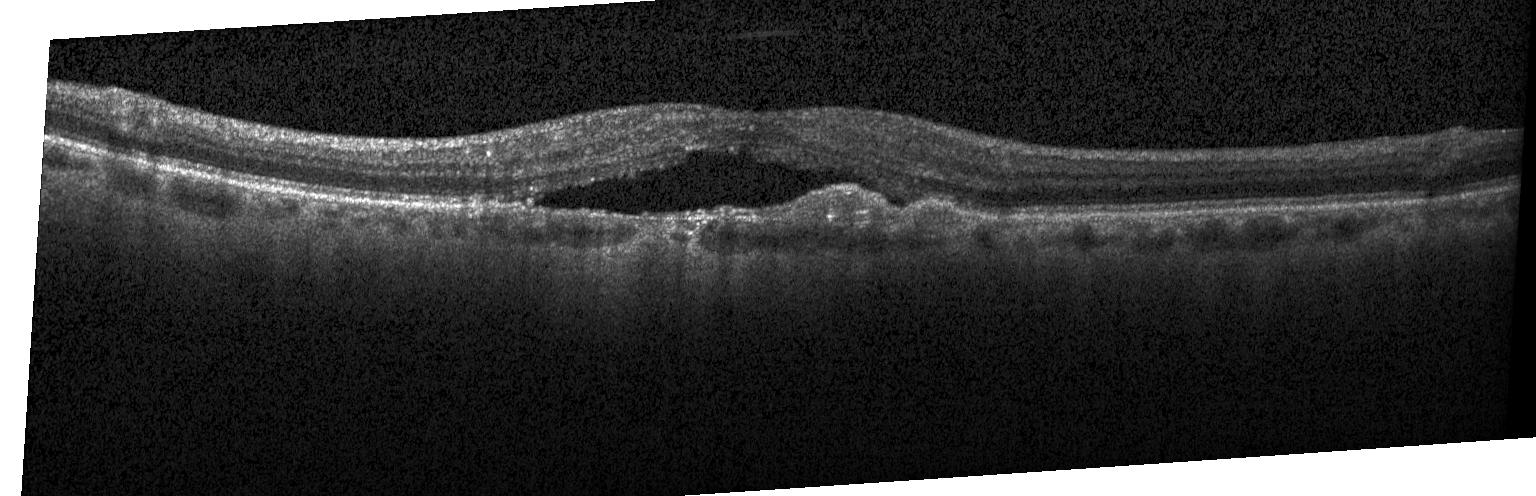

Spectral-domain OCT · optical coherence tomography B-scan. A choroidal neovascular membrane.